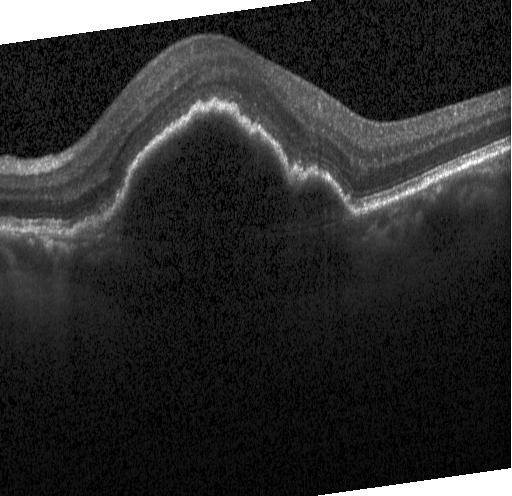
Spectral-domain optical coherence tomography · optical coherence tomography scan — Macular OCT: a choroidal neovascular membrane.